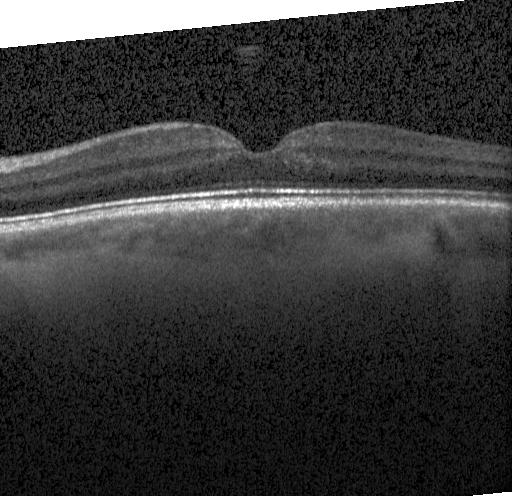
Impression: no CNV, no DME, and no drusen.